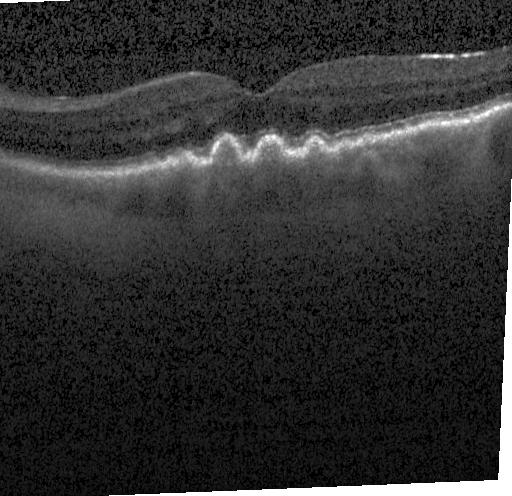
SD-OCT · OCT B-scan · Heidelberg Spectralis. Assessment: sub-RPE drusenoid deposits.